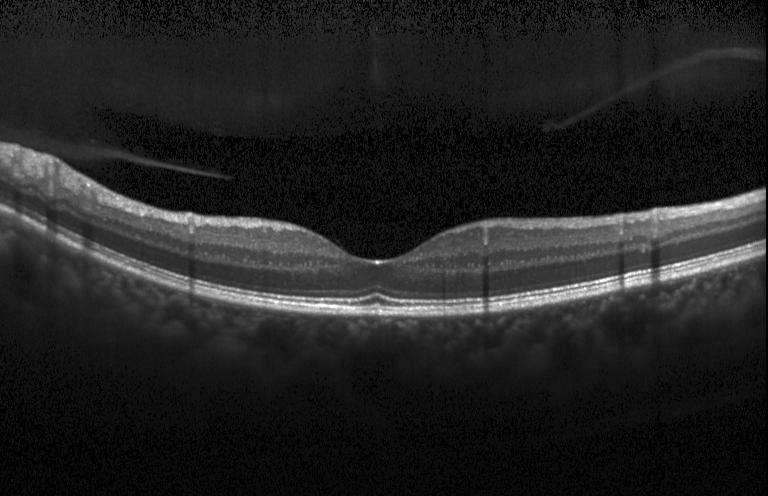
Through the macula. SD-OCT. Heidelberg Spectralis OCT system. Retinal OCT B-scan
Dx: neither CNV, DME, nor drusen.